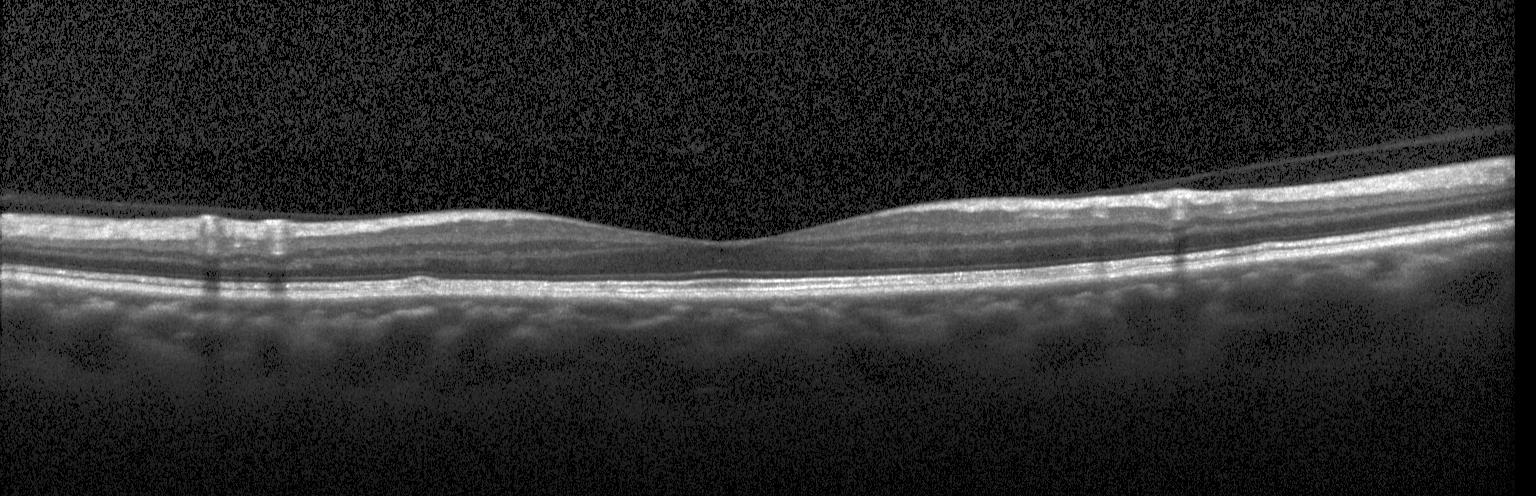 OCT scan showing no choroidal neovascularization, diabetic macular edema, or drusen.